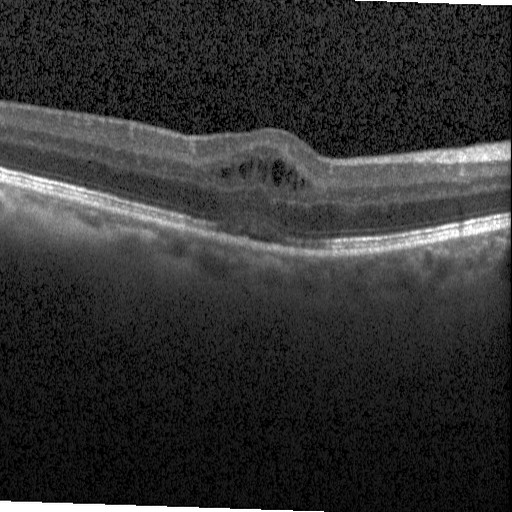
Retinal OCT cross-section.
Finding: diabetic macular edema.